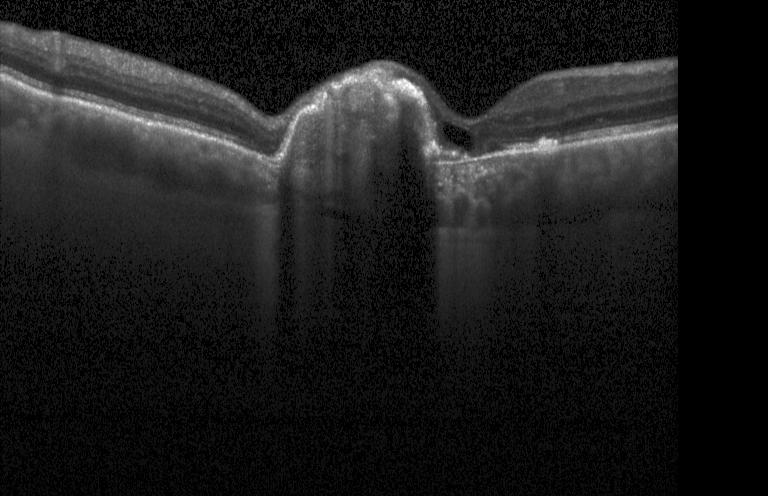 Spectral-domain OCT · centered on the fovea · optical coherence tomography scan · Heidelberg Spectralis
Choroidal neovascularization (CNV).